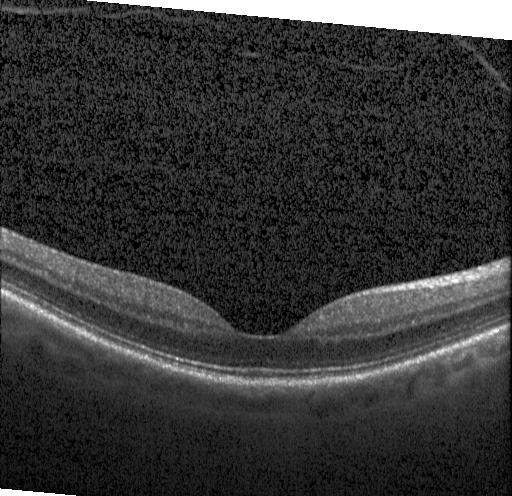

Optical coherence tomography scan
This B-scan demonstrates no choroidal neovascularization, no diabetic macular edema, and no drusen.